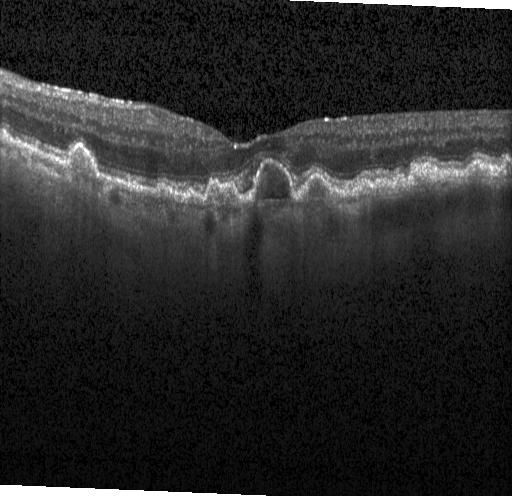
OCT line scan — The scan shows multiple drusen.